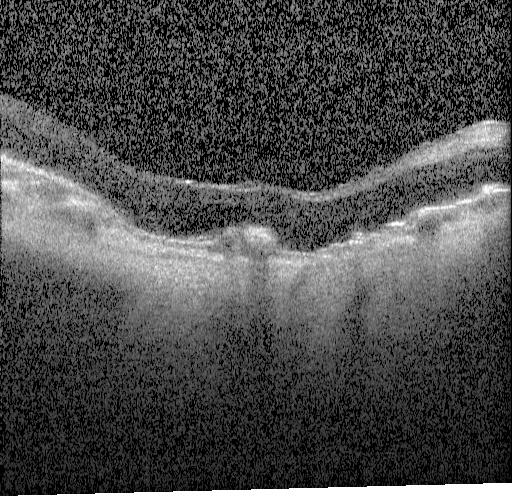
Retinal OCT B-scan. Spectral-domain optical coherence tomography — Assessment: a choroidal neovascular membrane.